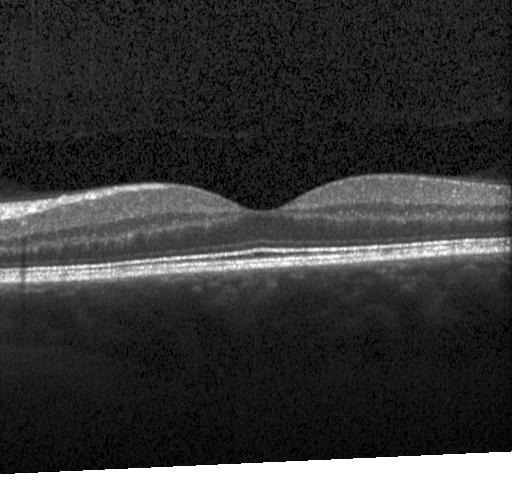
Retinal OCT B-scan
The scan shows no evidence of choroidal neovascularization, diabetic macular edema, or drusen.